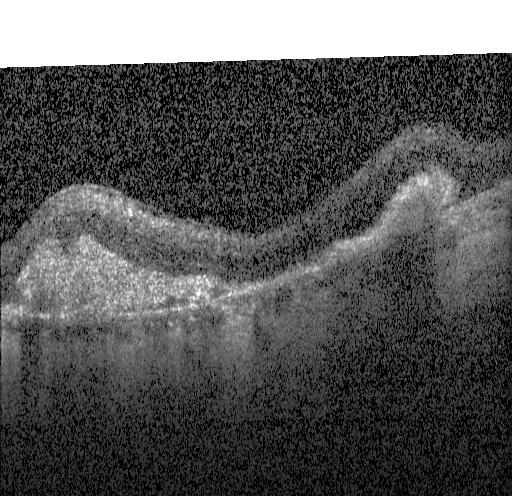 Spectral-domain OCT B-scan: choroidal neovascularization.